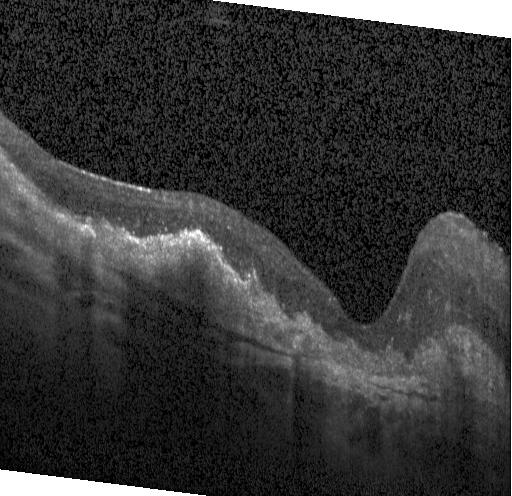
Spectral-domain OCT; optical coherence tomography B-scan
Impression: choroidal neovascularization.